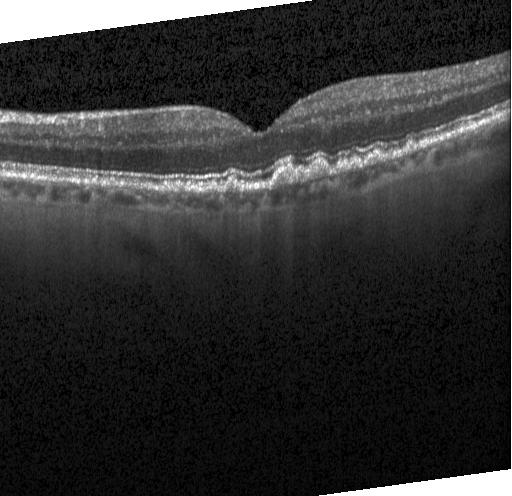

Finding: sub-RPE drusenoid deposits.